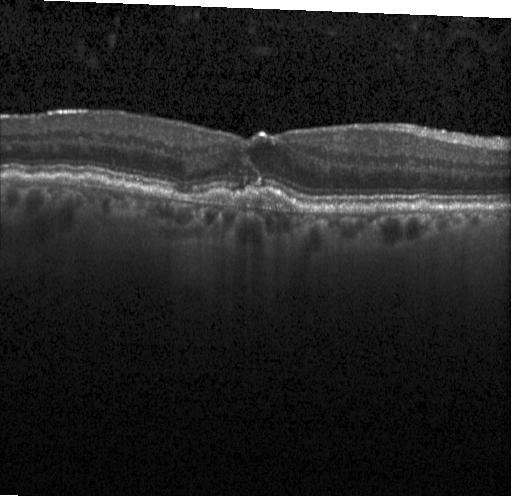 Macular OCT: a choroidal neovascular membrane.